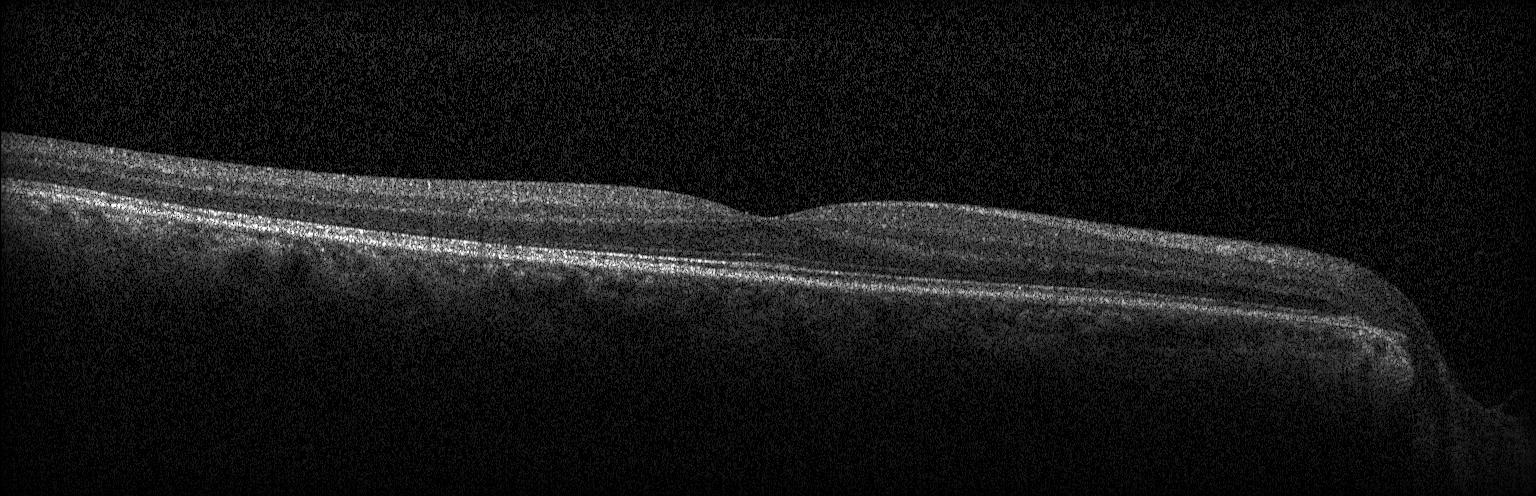

Heidelberg Spectralis OCT system; horizontal scan through the fovea; OCT line scan; spectral-domain OCT. Assessment: no evidence of choroidal neovascularization, diabetic macular edema, or drusen.